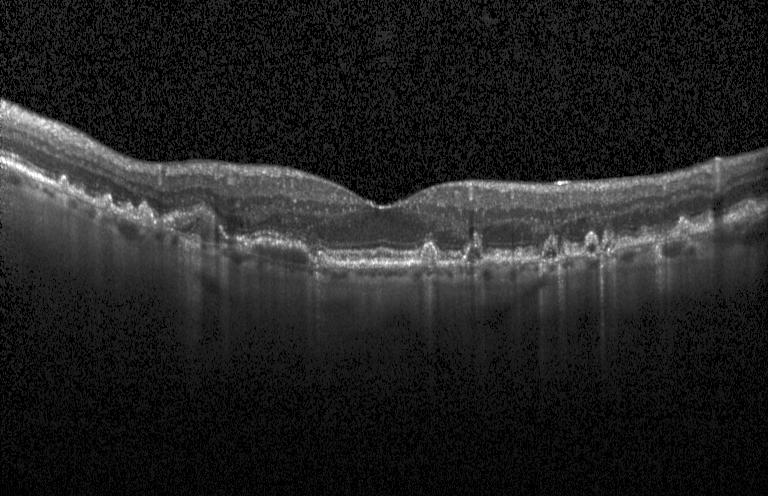
Optical coherence tomography scan, instrument: Heidelberg Spectralis, SD-OCT, centered on the fovea.
Macular OCT: choroidal neovascularization (CNV).